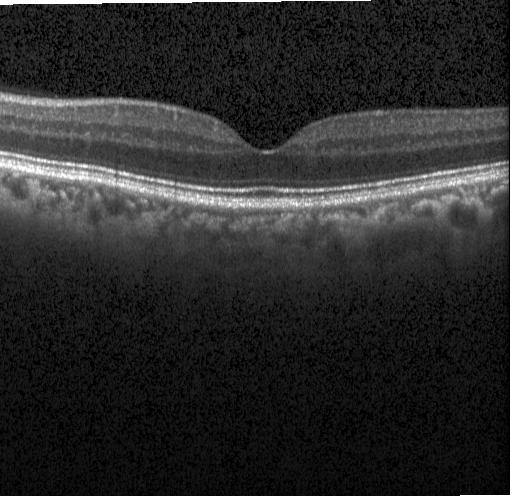
Spectral-domain optical coherence tomography; optical coherence tomography B-scan. OCT finding: no choroidal neovascularization, no diabetic macular edema, and no drusen.